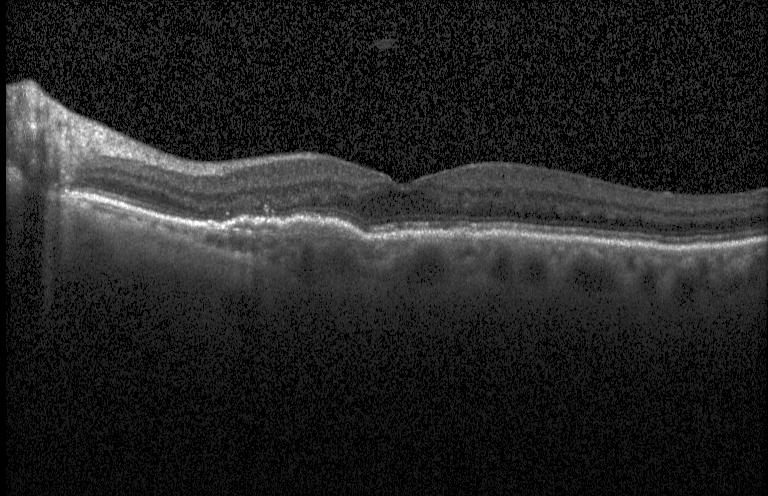 Assessment: CNV.